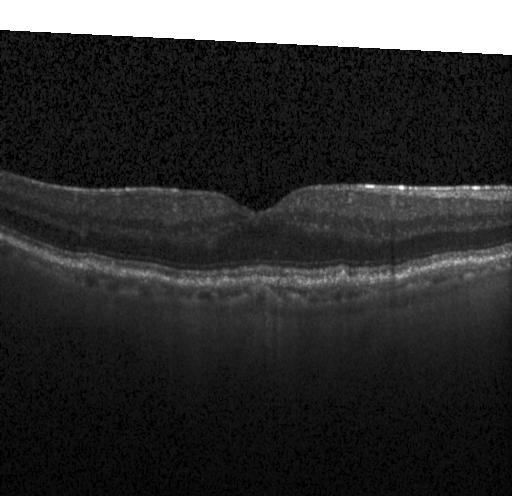

Optical coherence tomography scan — Dx: multiple drusen.